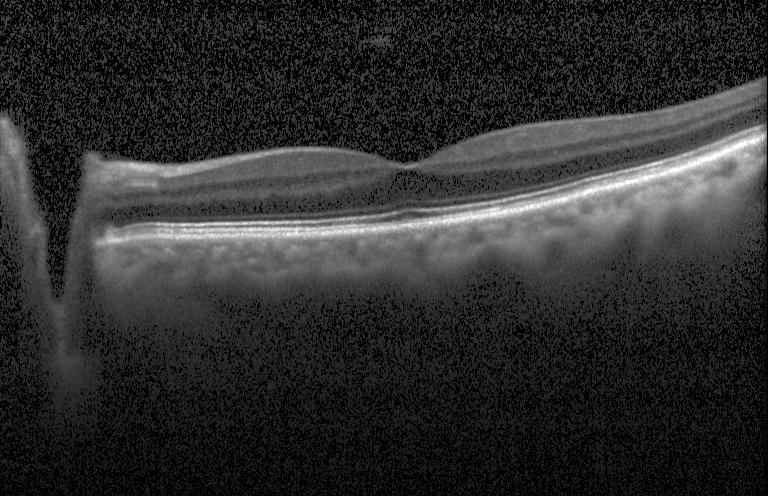

Optical coherence tomography scan, spectral-domain optical coherence tomography, through the macula — Macular OCT: no choroidal neovascularization, no diabetic macular edema, and no drusen.